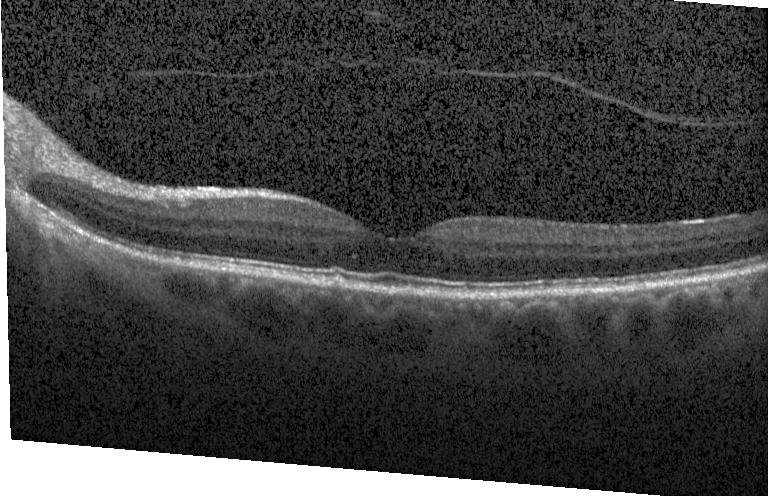 Impression: drusen.